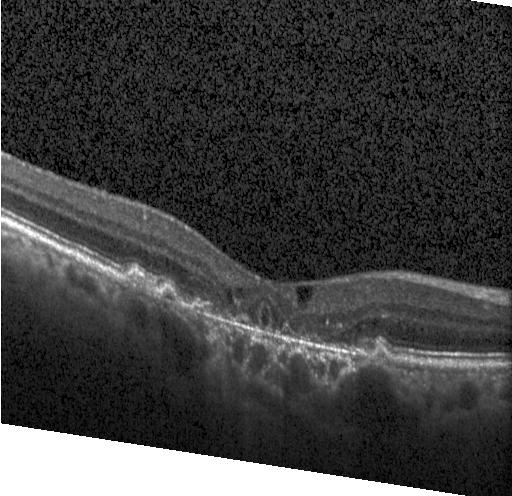

Spectral-domain optical coherence tomography. Optical coherence tomography scan.
Macular OCT: choroidal neovascularization.